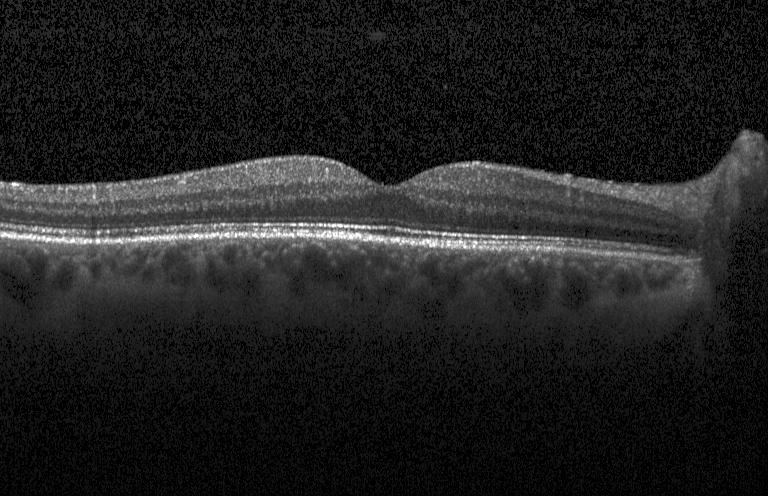
Assessment: no evidence of choroidal neovascularization, diabetic macular edema, or drusen.